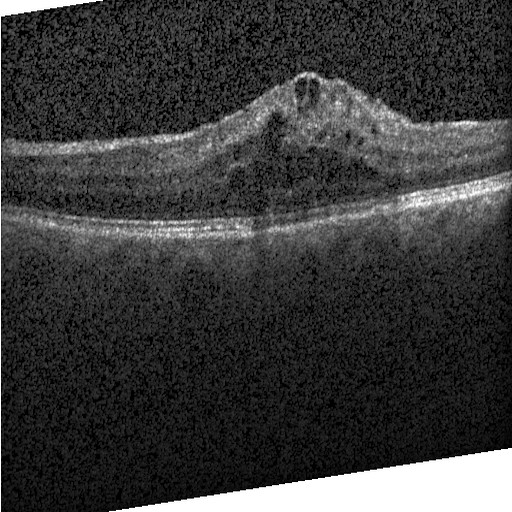 Optical coherence tomography B-scan
Diagnosis: DME.